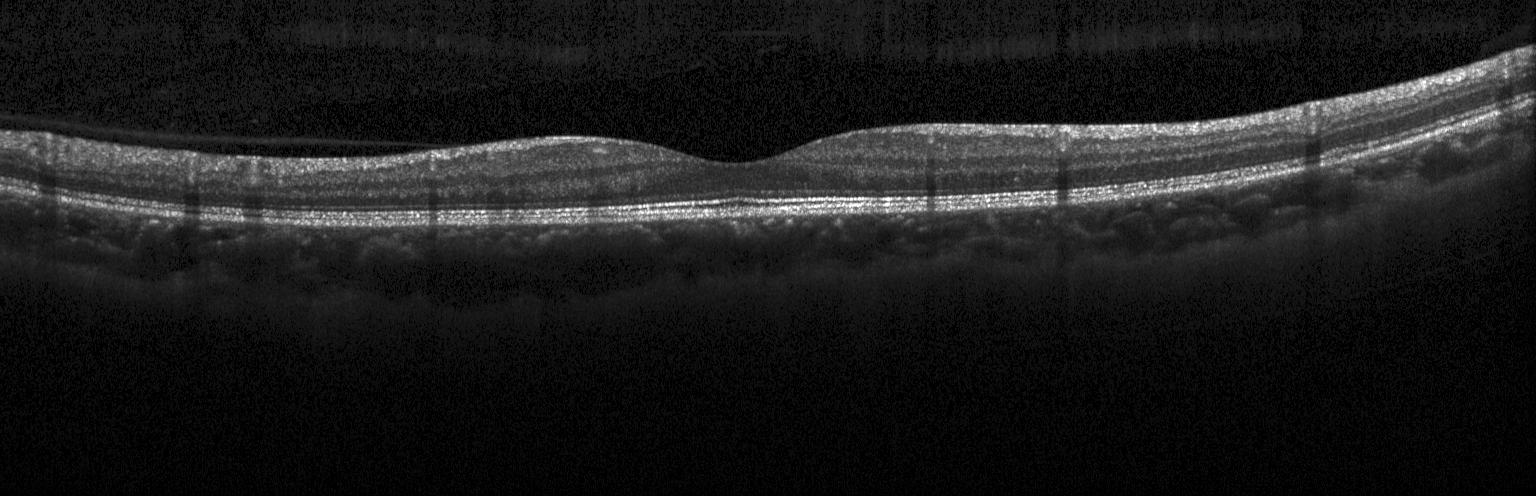
Retinal OCT B-scan.
Dx: no evidence of CNV, DME, or drusen.